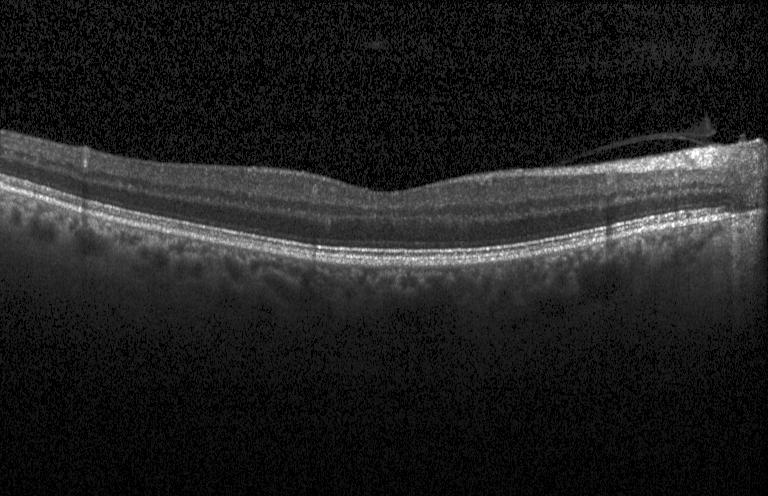 Heidelberg Spectralis OCT system, SD-OCT, retinal OCT B-scan.
Finding: no evidence of choroidal neovascularization, diabetic macular edema, or drusen.